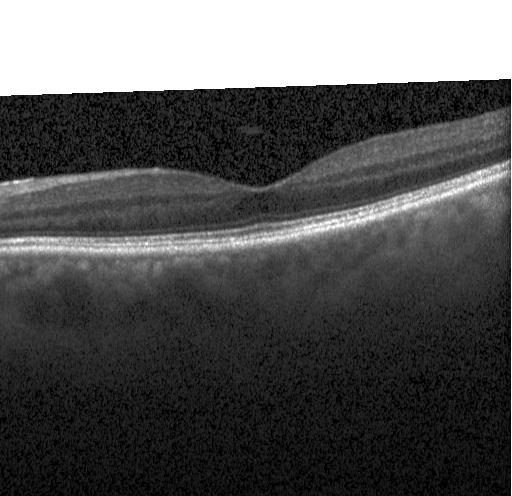

Impression: no CNV, DME, or drusen.